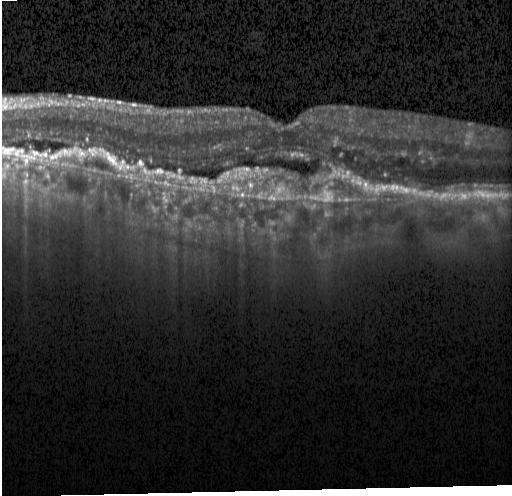
Retinal OCT cross-section. OCT finding: choroidal neovascularization (CNV).